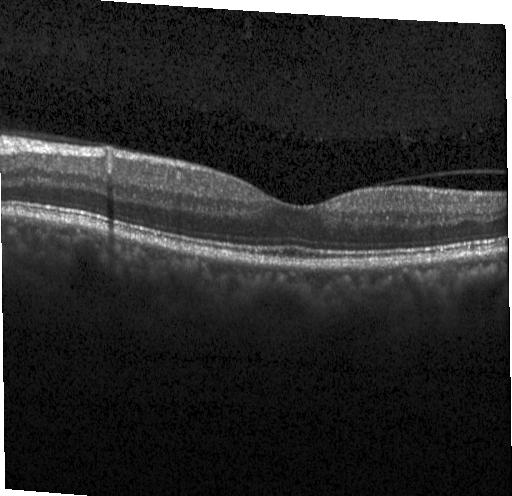 OCT finding: neither CNV, DME, nor drusen.